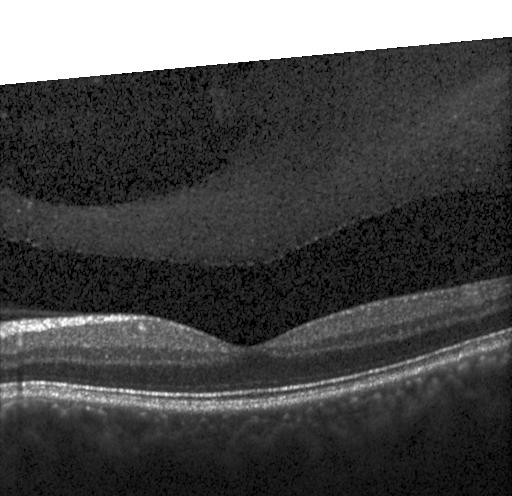

Optical coherence tomography scan.
Finding: neither choroidal neovascularization, diabetic macular edema, nor drusen.